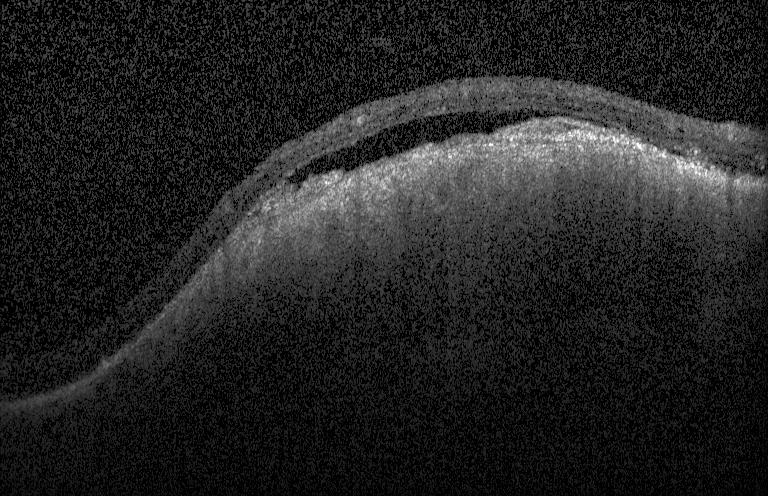

Instrument: Heidelberg Spectralis · retinal OCT cross-section · centered on the fovea.
Diagnosis: a choroidal neovascular membrane.